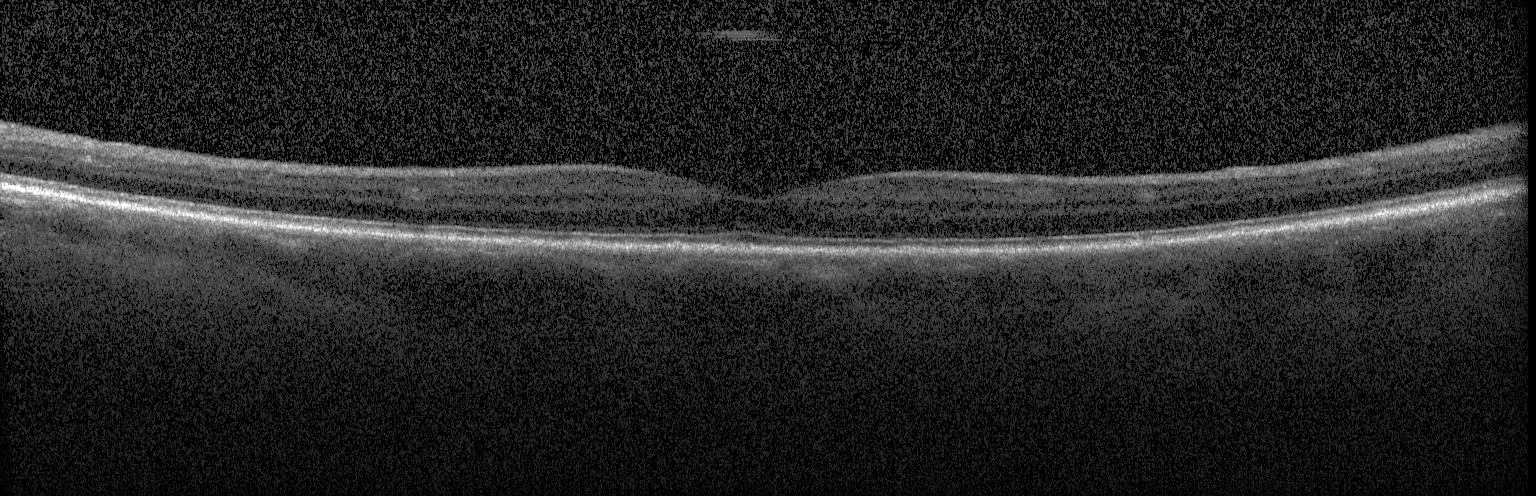

No evidence of choroidal neovascularization, diabetic macular edema, or drusen.